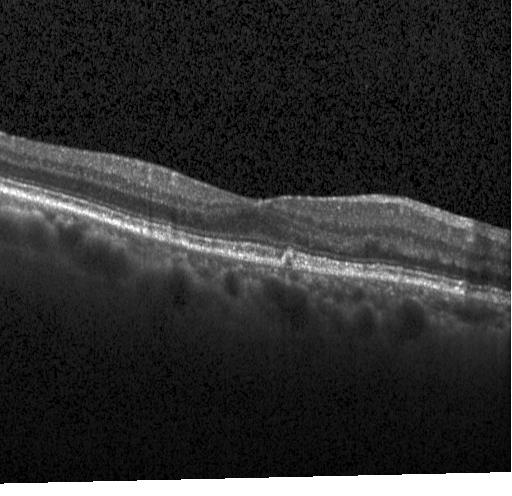
Finding: drusen.